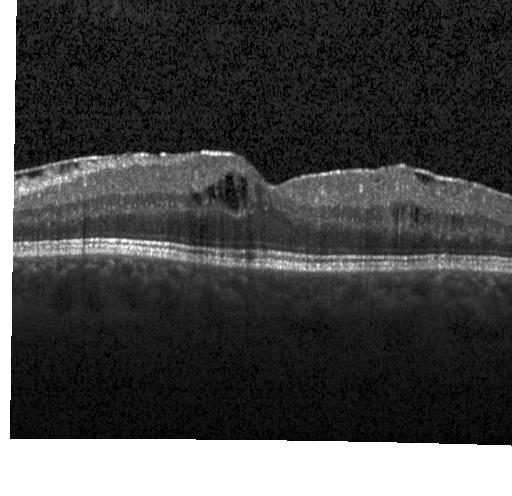 Optical coherence tomography scan. Horizontal scan through the fovea. Spectral-domain optical coherence tomography.
The scan shows diabetic macular edema (DME).